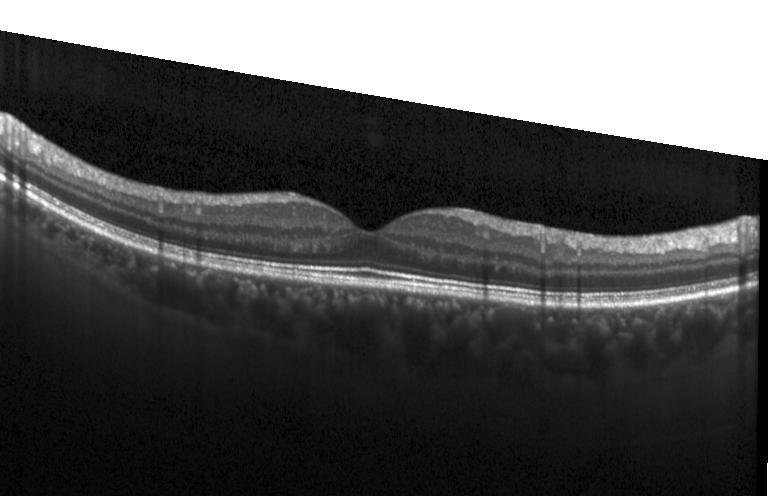

OCT finding: no CNV, no DME, and no drusen.